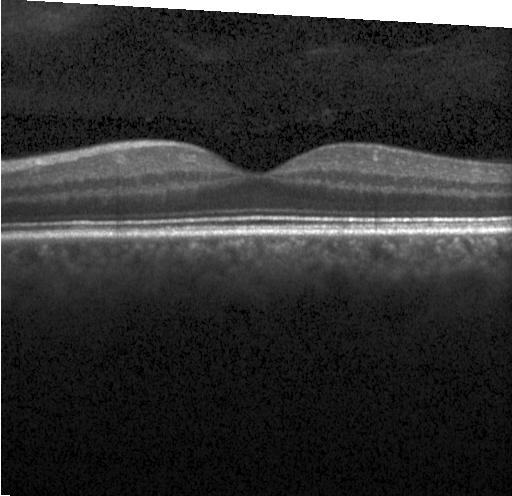

The scan shows no evidence of CNV, DME, or drusen.